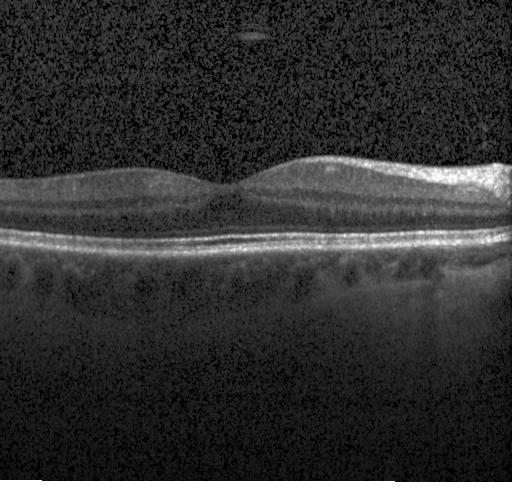 Spectral-domain OCT, retinal OCT cross-section, through the macula — Impression: neither CNV, DME, nor drusen.